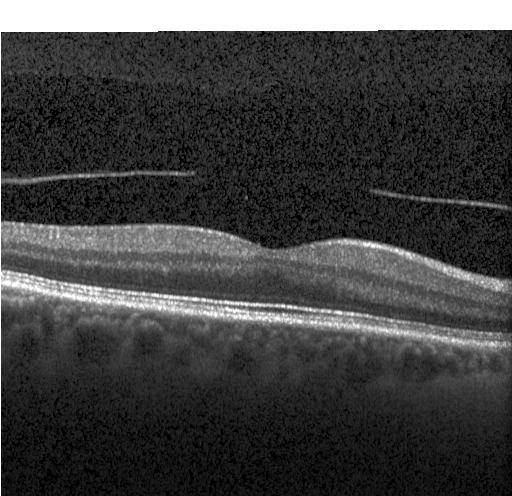

Retinal OCT cross-section
Finding: neither choroidal neovascularization, diabetic macular edema, nor drusen.